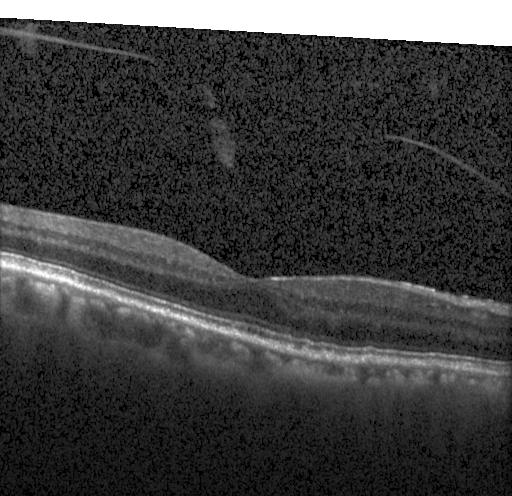

SD-OCT. Optical coherence tomography scan. Diagnosis: multiple drusen.